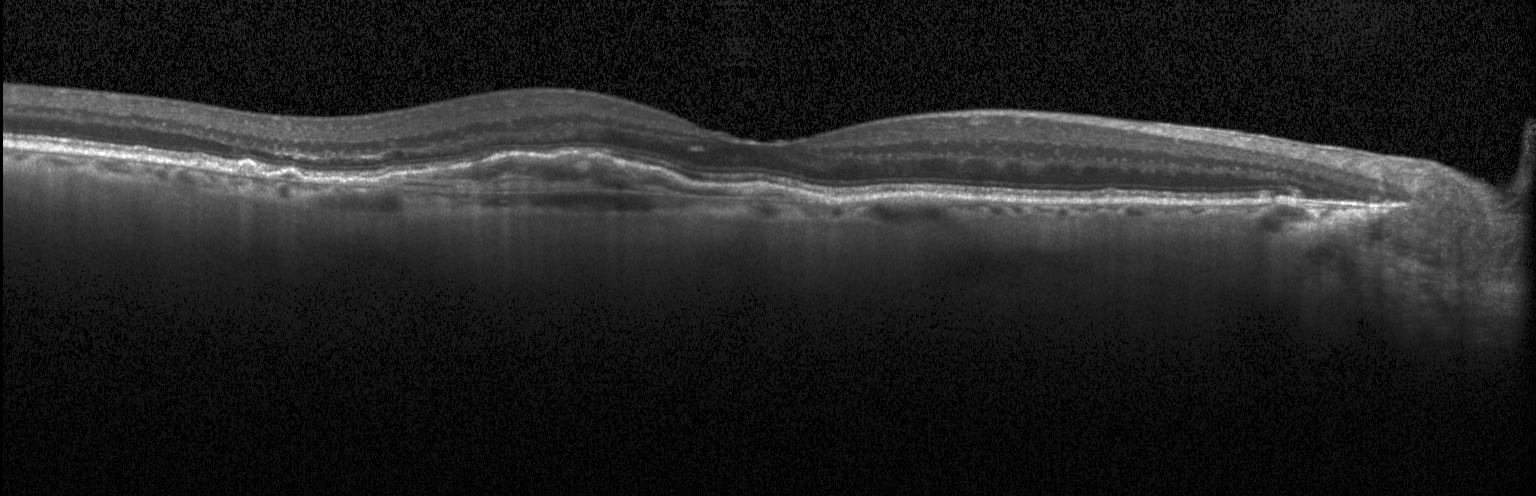
Assessment: CNV.